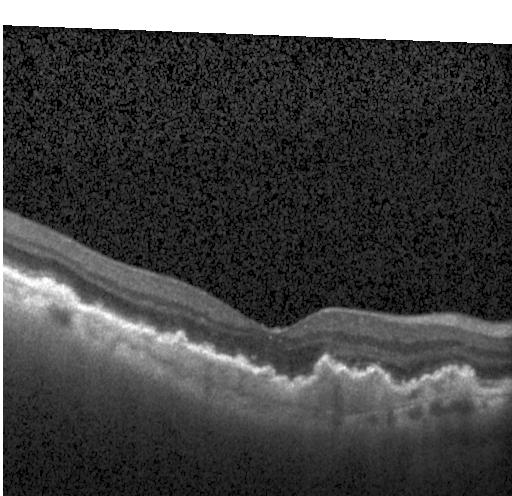
Optical coherence tomography scan. Heidelberg Spectralis OCT system.
Finding: a choroidal neovascular membrane.